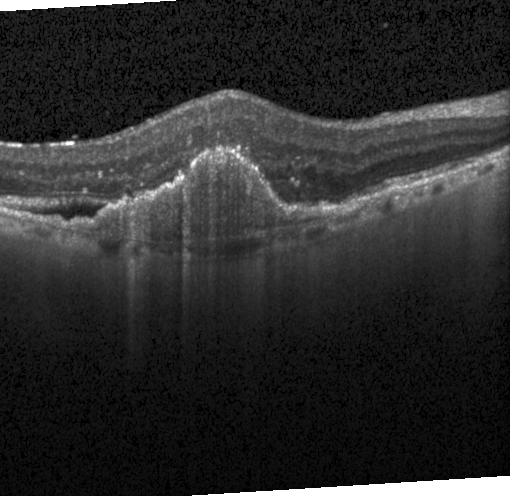

Centered on the fovea · Heidelberg Spectralis OCT system · retinal OCT cross-section. OCT finding: a choroidal neovascular membrane.